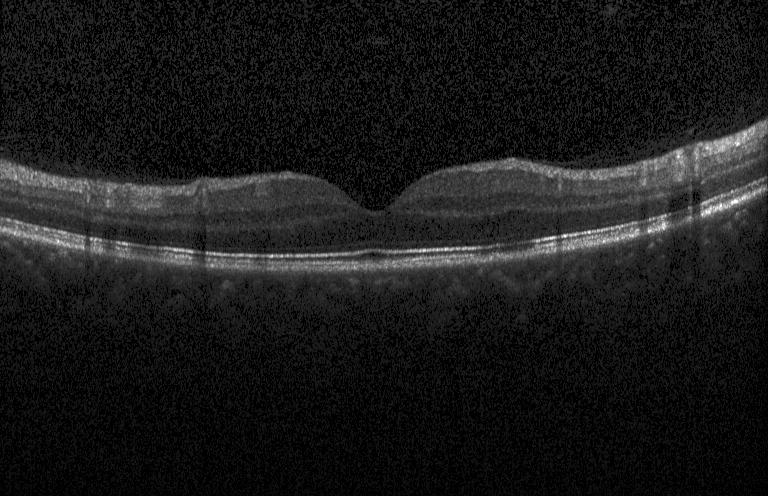 Spectral-domain optical coherence tomography, fovea-centered, retinal OCT B-scan, acquired on a Heidelberg Spectralis. Diagnosis: no CNV, no DME, and no drusen.